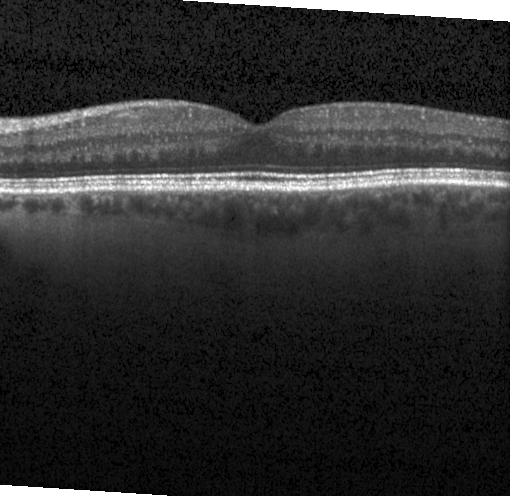 Impression: no CNV, DME, or drusen.